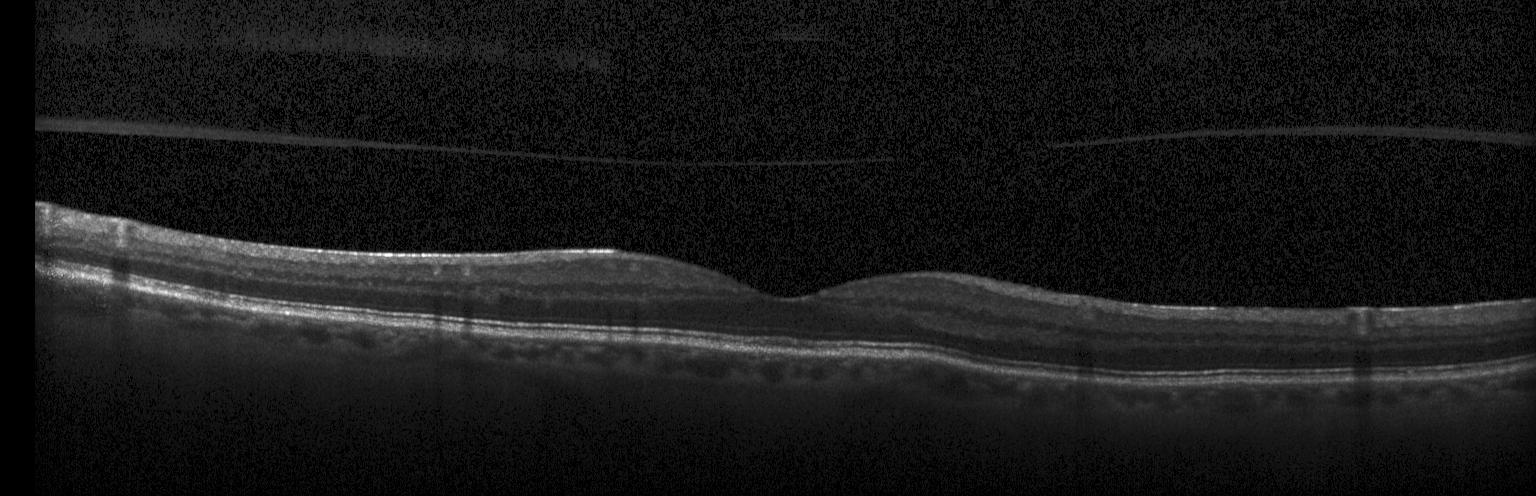 Instrument: Heidelberg Spectralis · optical coherence tomography B-scan · SD-OCT — OCT finding: no choroidal neovascularization, diabetic macular edema, or drusen.